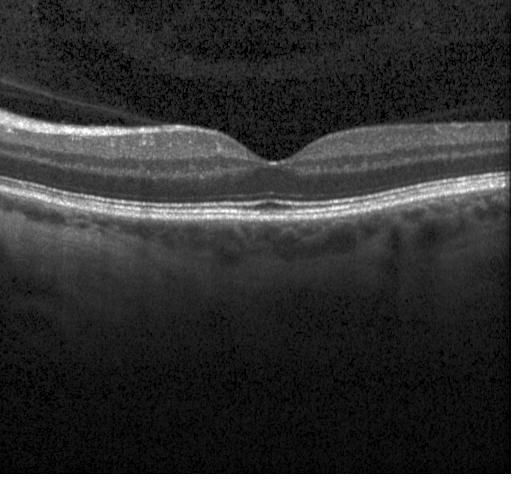 SD-OCT. OCT line scan — Diagnosis: no choroidal neovascularization, no diabetic macular edema, and no drusen.